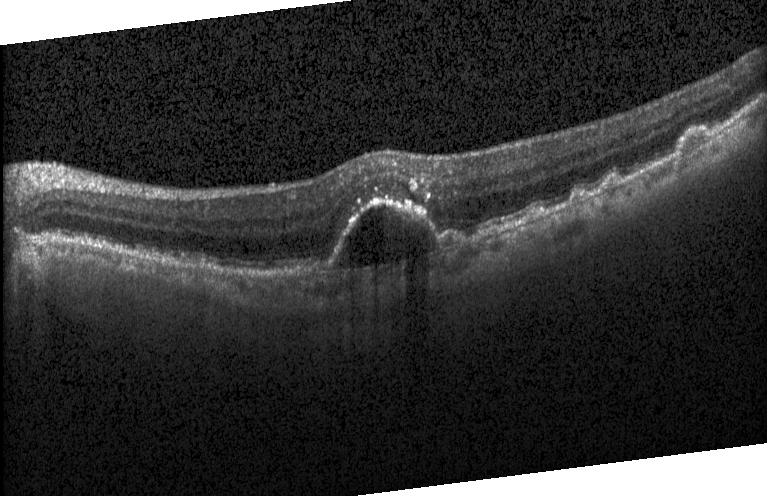 OCT line scan
Diagnosis: CNV.